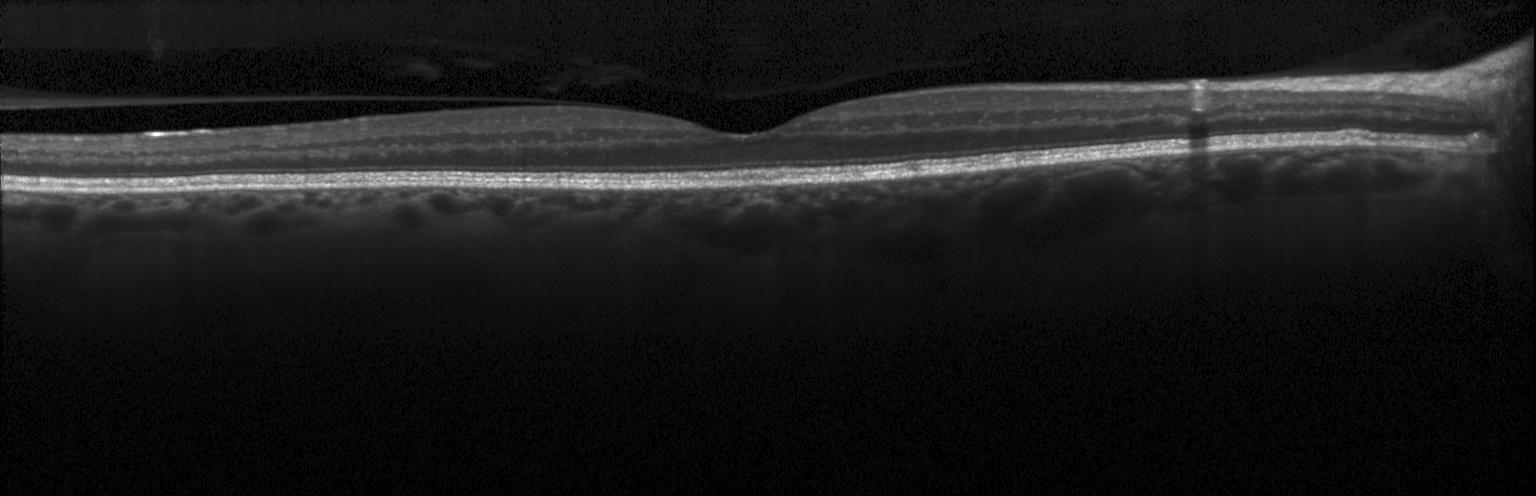

Spectral-domain optical coherence tomography · optical coherence tomography B-scan · instrument: Heidelberg Spectralis · macular scan — Diagnosis: no CNV, DME, or drusen.